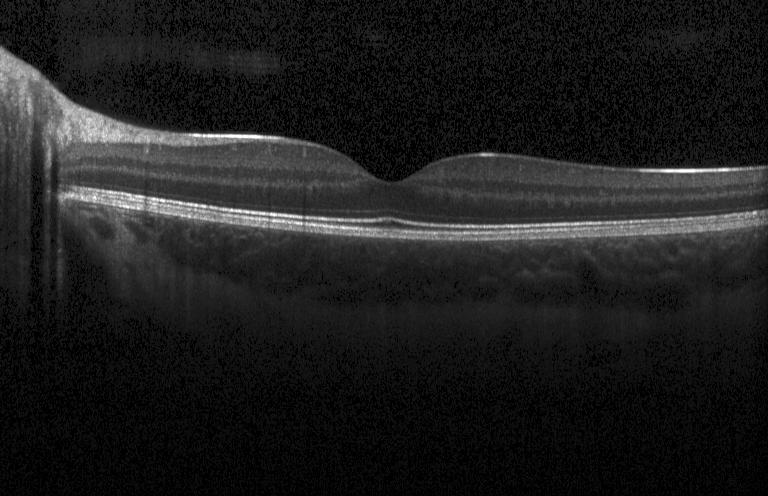 Optical coherence tomography B-scan. Dx: no evidence of choroidal neovascularization, diabetic macular edema, or drusen.